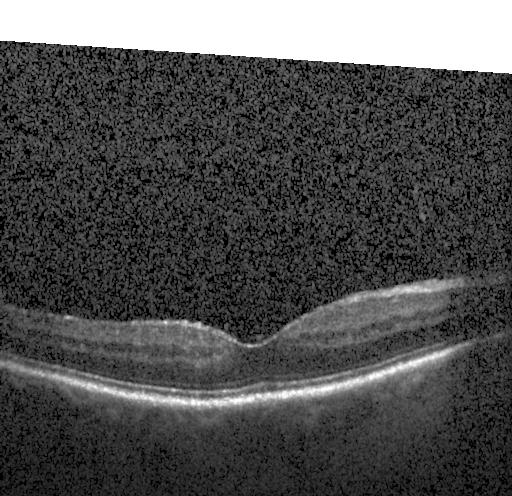

OCT line scan · SD-OCT · instrument: Heidelberg Spectralis
Macular OCT: no CNV, no DME, and no drusen.